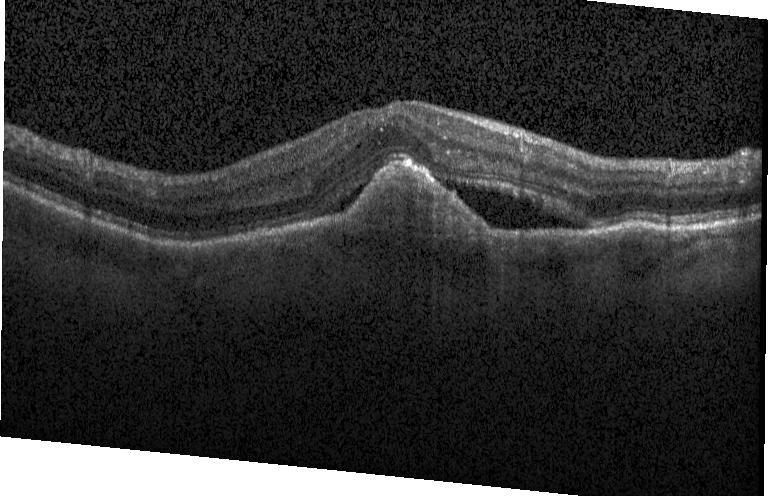 Retinal OCT cross-section; spectral-domain optical coherence tomography
A choroidal neovascular membrane.